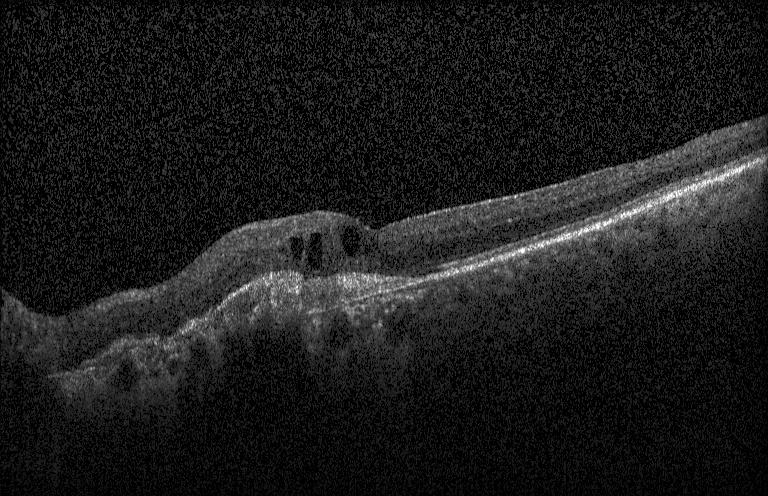 OCT finding: a choroidal neovascular membrane.